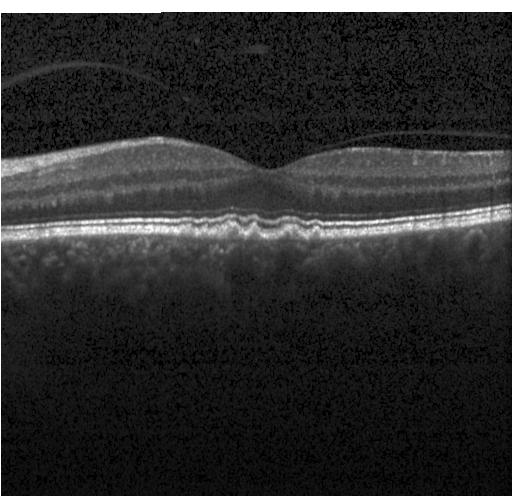

Through the macula. Optical coherence tomography B-scan. Spectral-domain OCT — Finding: sub-RPE drusenoid deposits.